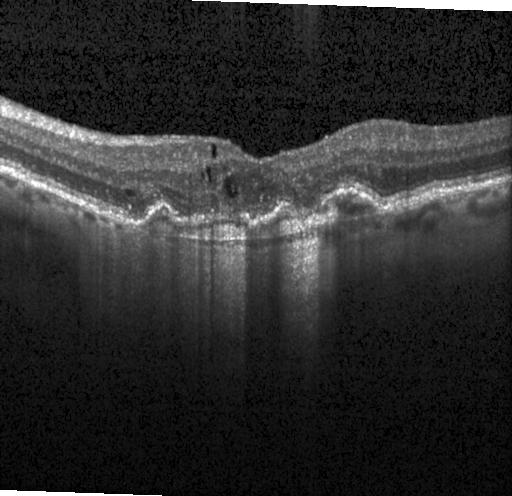
Diagnosis: a choroidal neovascular membrane.